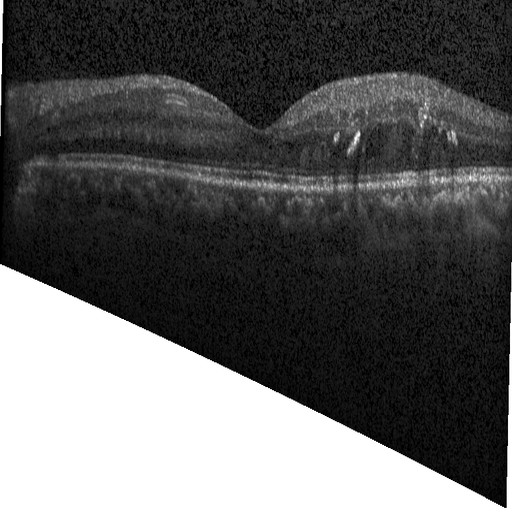 Impression: diabetic macular edema.